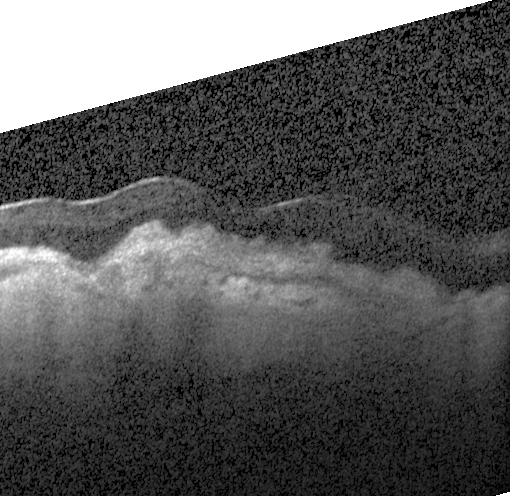
Retinal OCT cross-section showing choroidal neovascularization (CNV).